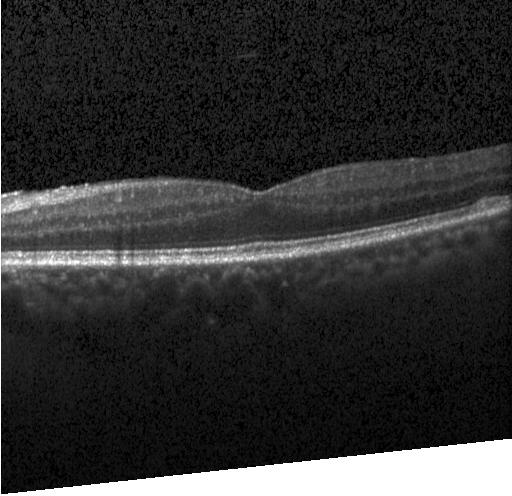 Macular OCT demonstrating no choroidal neovascularization, no diabetic macular edema, and no drusen.